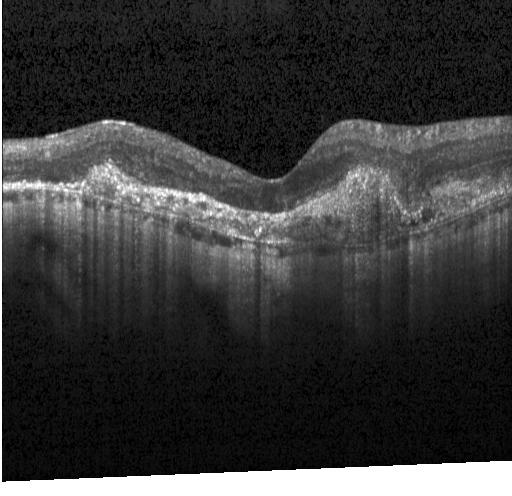
Centered on the fovea; Heidelberg Spectralis; OCT line scan; spectral-domain optical coherence tomography
Finding: CNV.